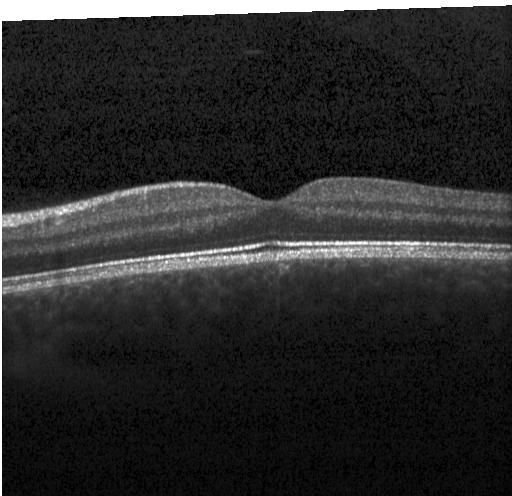

Spectral-domain OCT · macular scan · optical coherence tomography B-scan · Heidelberg Spectralis
Dx: no choroidal neovascularization, no diabetic macular edema, and no drusen.